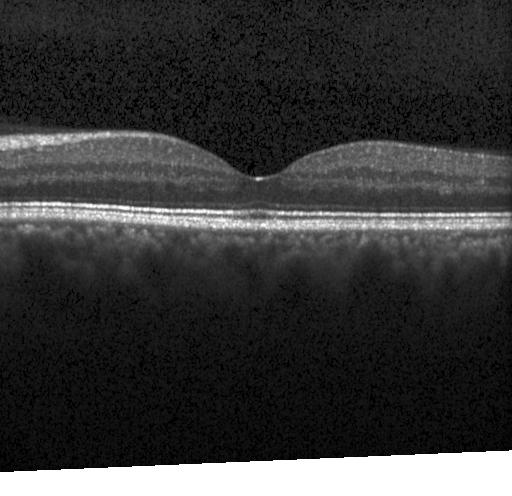
This B-scan demonstrates no CNV, DME, or drusen.